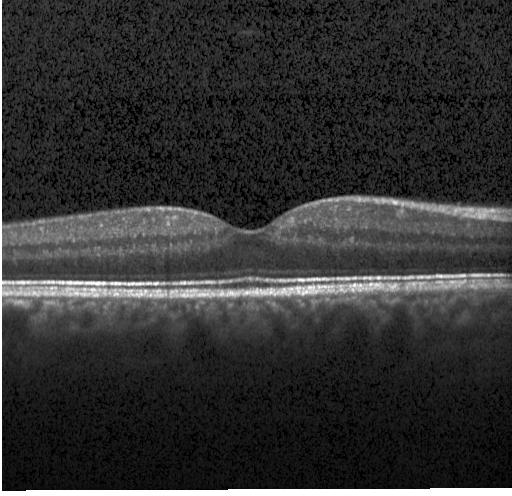 Centered on the fovea. Optical coherence tomography scan
Dx: no choroidal neovascularization, diabetic macular edema, or drusen.